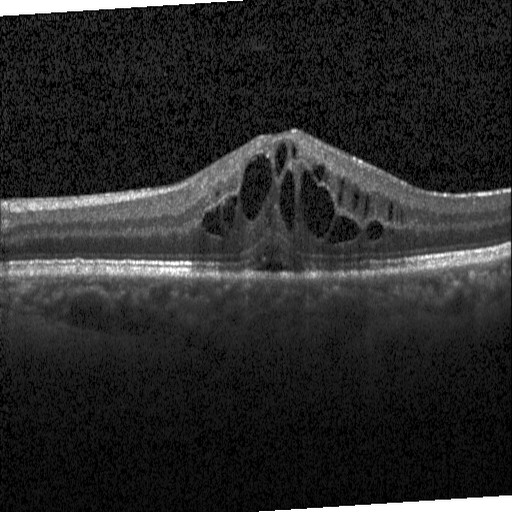

Retinal OCT B-scan; horizontal scan through the fovea. DME.